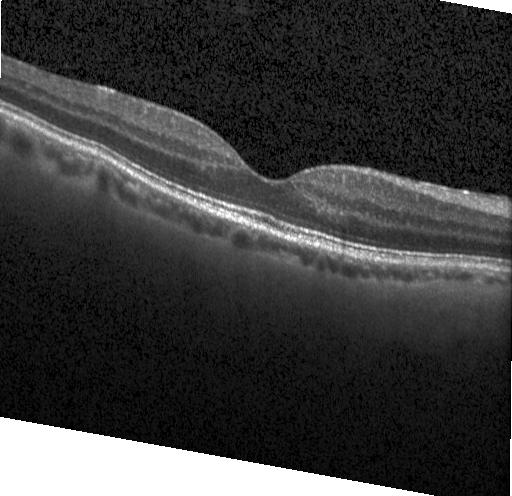 Retinal OCT cross-section — Macular OCT: no choroidal neovascularization, diabetic macular edema, or drusen.